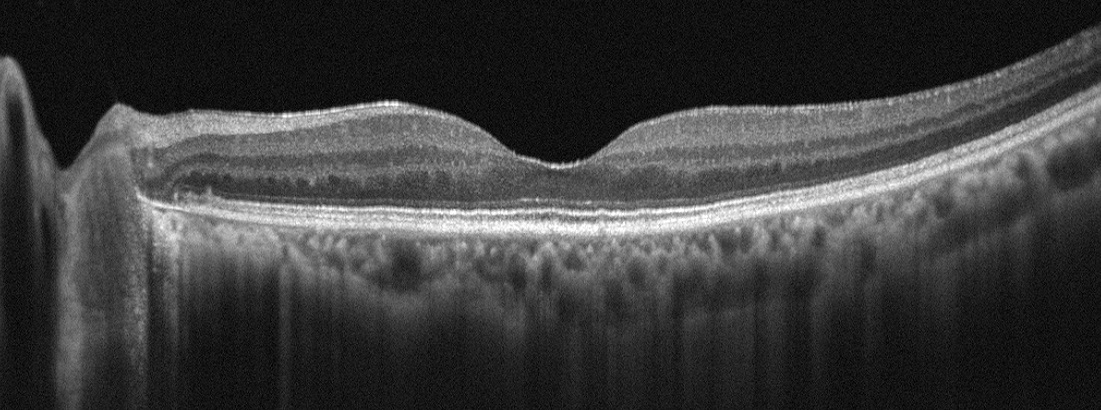 Finding: age-related macular degeneration (AMD).